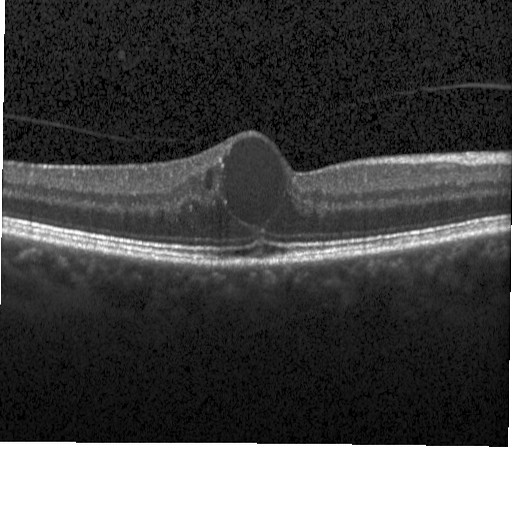 OCT line scan. Spectral-domain optical coherence tomography. Centered on the fovea
Diagnosis: diabetic macular edema.